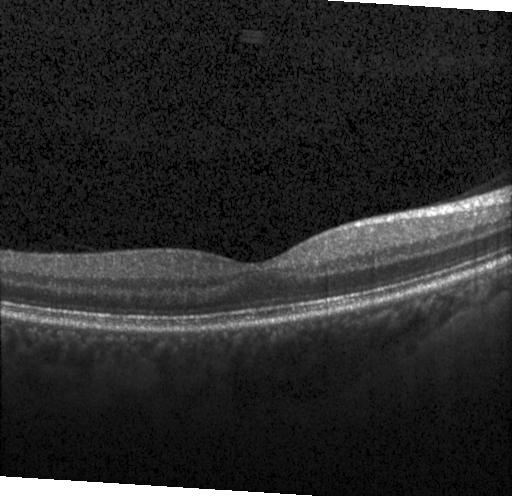
OCT line scan, spectral-domain optical coherence tomography — The scan shows no evidence of CNV, DME, or drusen.